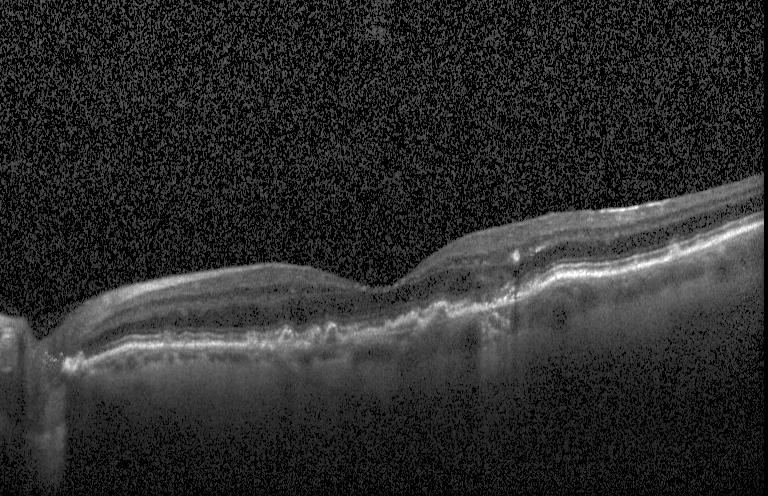
OCT B-scan.
Impression: multiple drusen.